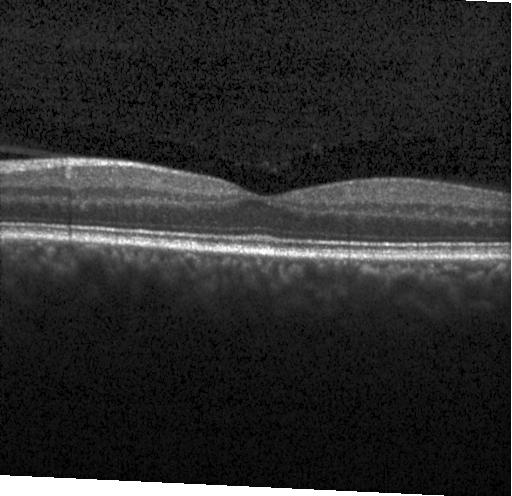
Horizontal scan through the fovea; instrument: Heidelberg Spectralis; optical coherence tomography scan; spectral-domain OCT.
Diagnosis: no CNV, no DME, and no drusen.